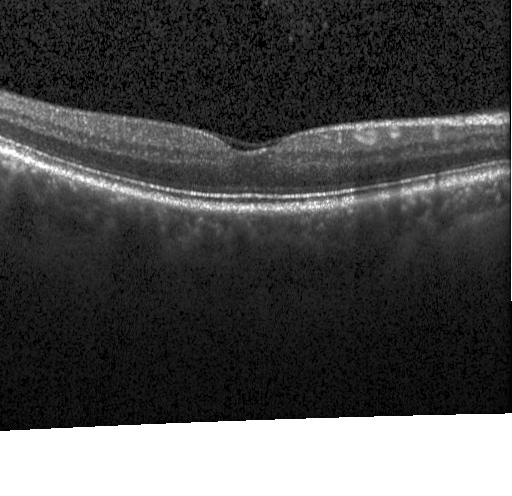

Macular OCT demonstrating neither choroidal neovascularization, diabetic macular edema, nor drusen.